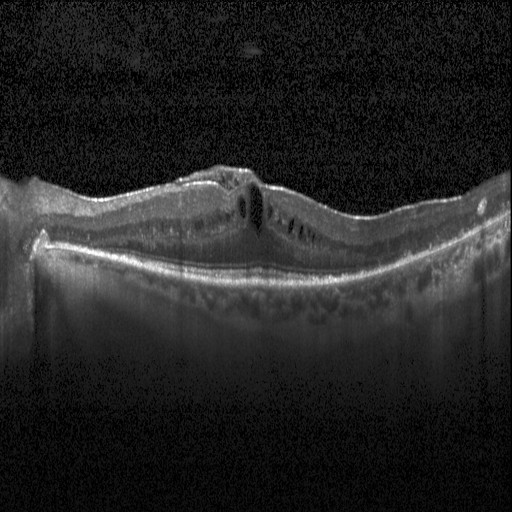

Macular OCT demonstrating DME.